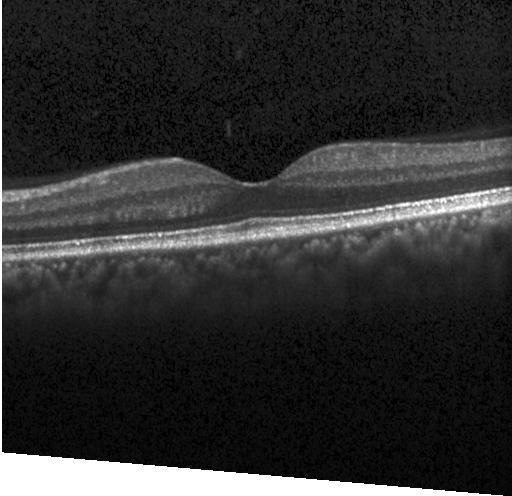

Optical coherence tomography scan; acquired on a Heidelberg Spectralis. Impression: no evidence of CNV, DME, or drusen.